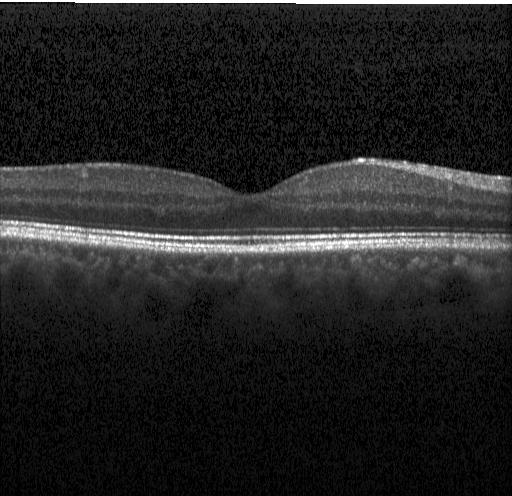 Acquired on a Heidelberg Spectralis; OCT line scan; SD-OCT; through the macula. Diagnosis: neither choroidal neovascularization, diabetic macular edema, nor drusen.